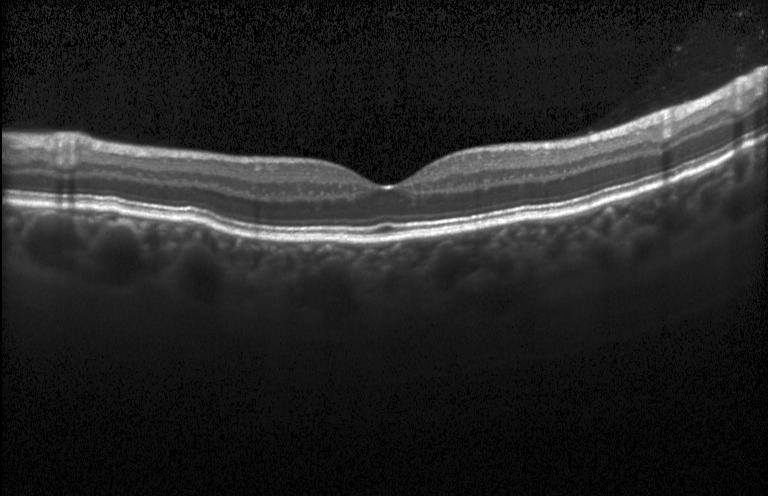
Diagnosis: no evidence of CNV, DME, or drusen.